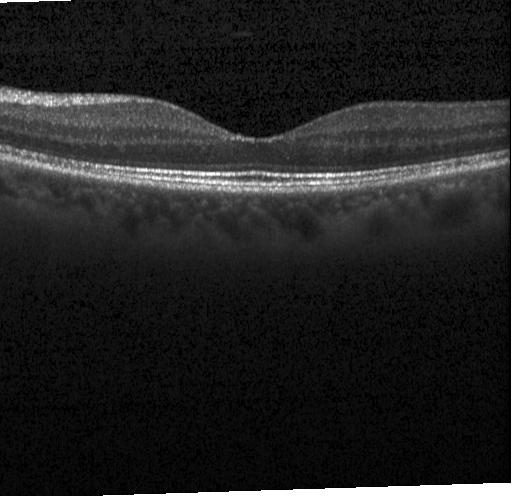
Fovea-centered. SD-OCT. Instrument: Heidelberg Spectralis. Optical coherence tomography B-scan
Finding: neither choroidal neovascularization, diabetic macular edema, nor drusen.